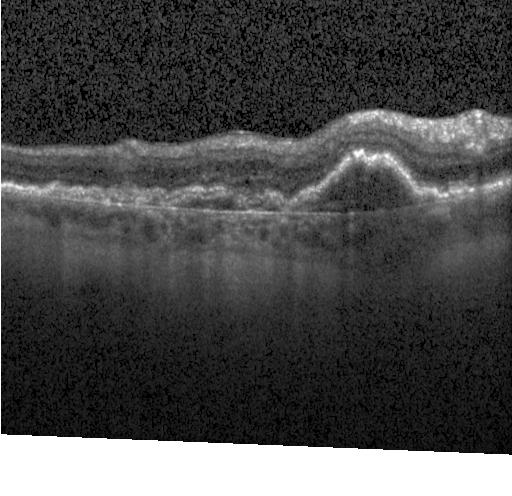

Optical coherence tomography scan; acquired on a Heidelberg Spectralis; SD-OCT; through the macula — Dx: a choroidal neovascular membrane.